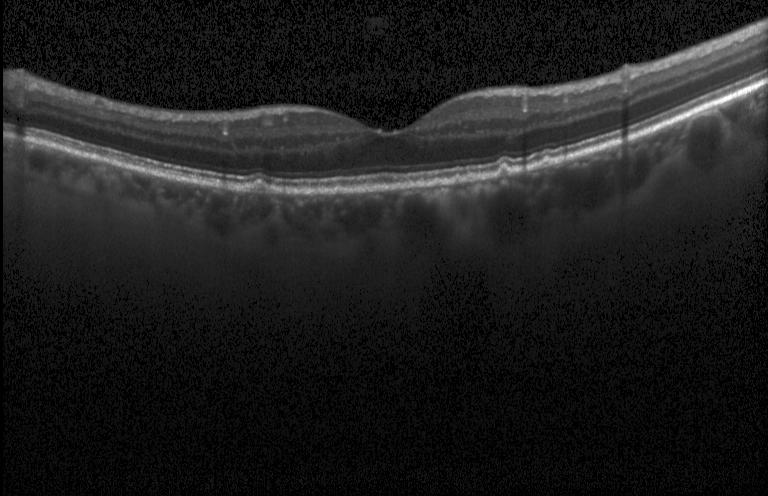 Spectral-domain OCT · optical coherence tomography scan · through the macula.
Assessment: sub-RPE drusenoid deposits.